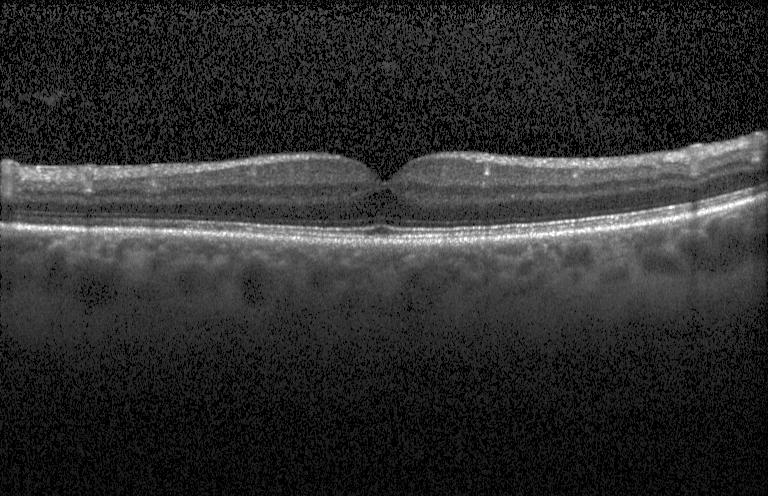
Retinal OCT B-scan. Finding: no choroidal neovascularization, no diabetic macular edema, and no drusen.